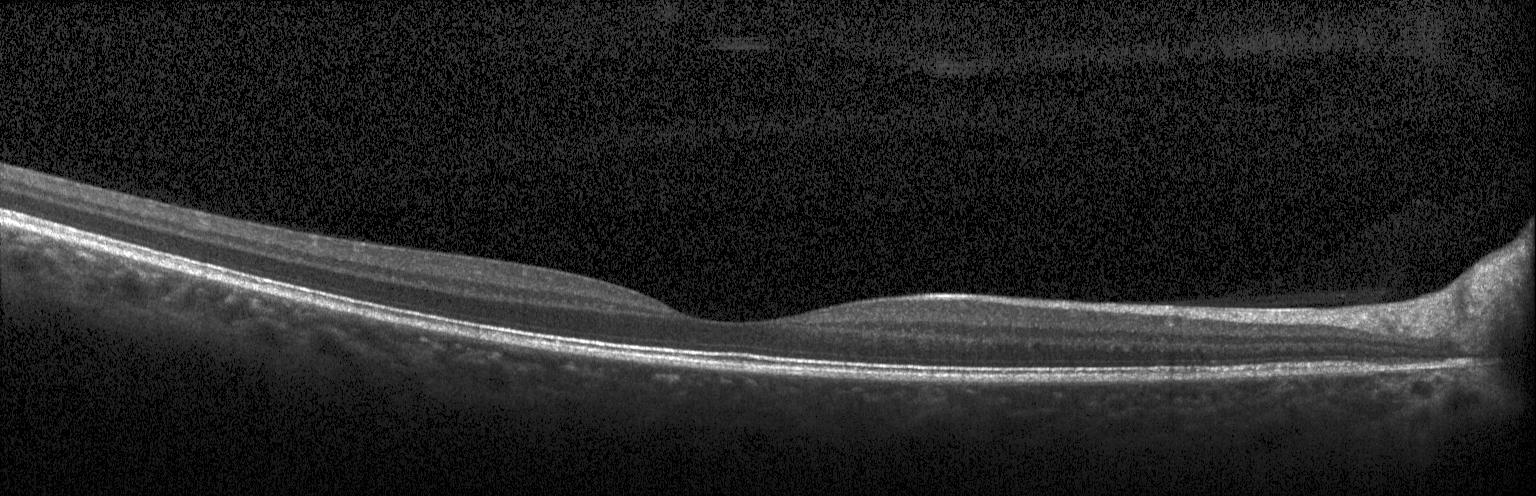
Macular OCT: no CNV, no DME, and no drusen.